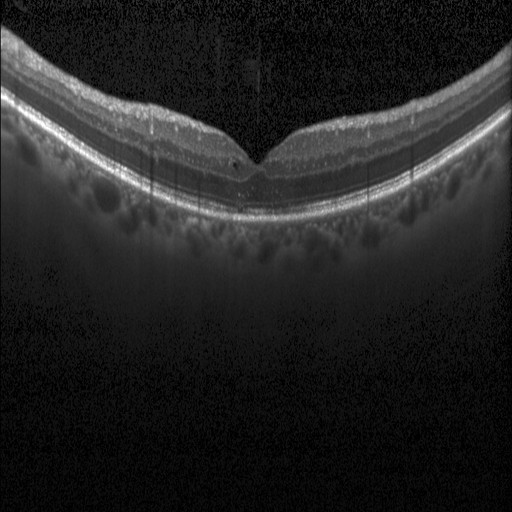 Horizontal scan through the fovea. Spectral-domain optical coherence tomography. Acquired on a Heidelberg Spectralis. Retinal OCT cross-section. Finding: DME.